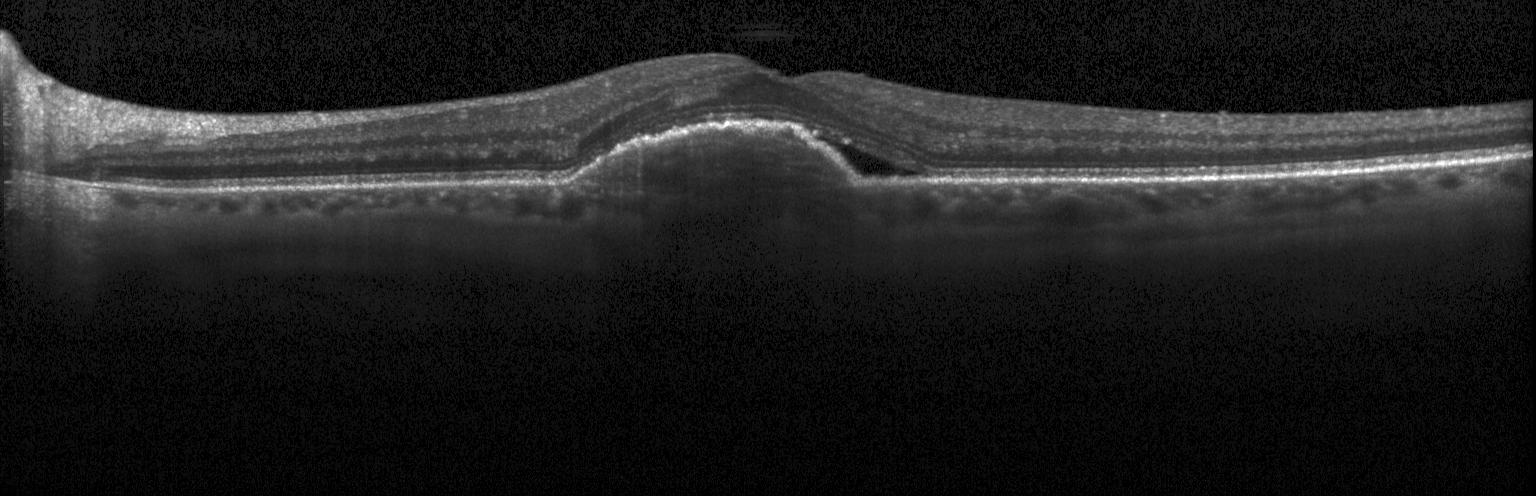
Fovea-centered. Retinal OCT B-scan. Instrument: Heidelberg Spectralis. Spectral-domain optical coherence tomography. This B-scan demonstrates CNV.